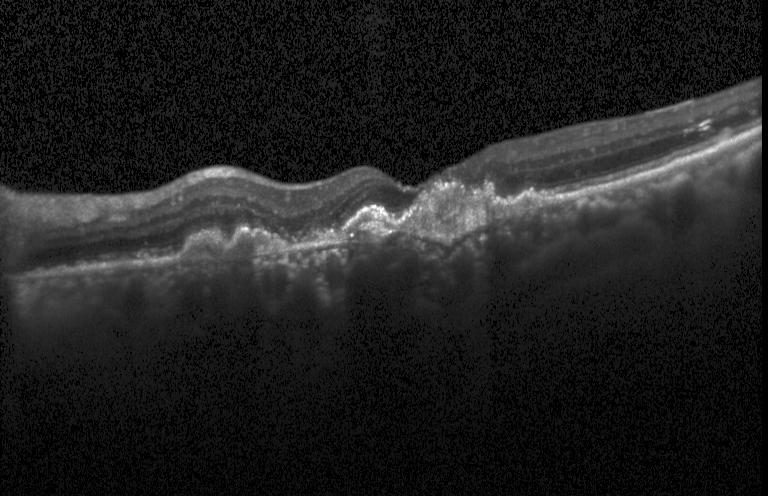 Retinal OCT B-scan; SD-OCT; fovea-centered — Diagnosis: a choroidal neovascular membrane.